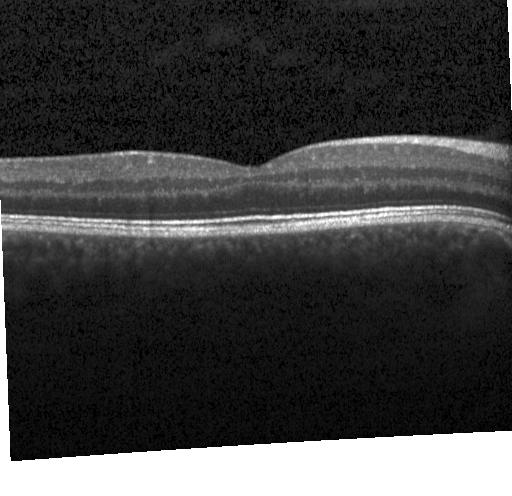
Spectral-domain OCT, optical coherence tomography B-scan. Impression: no choroidal neovascularization, diabetic macular edema, or drusen.